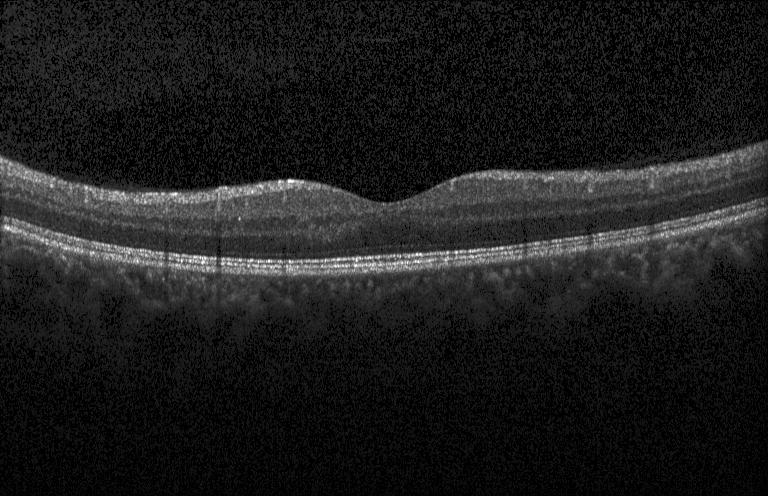 OCT line scan. Acquired on a Heidelberg Spectralis. SD-OCT. Fovea-centered — Assessment: no CNV, DME, or drusen.